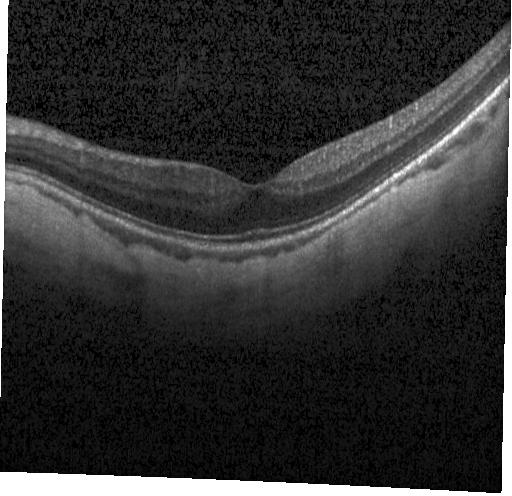
Instrument: Heidelberg Spectralis, spectral-domain optical coherence tomography, optical coherence tomography B-scan
Impression: no evidence of CNV, DME, or drusen.